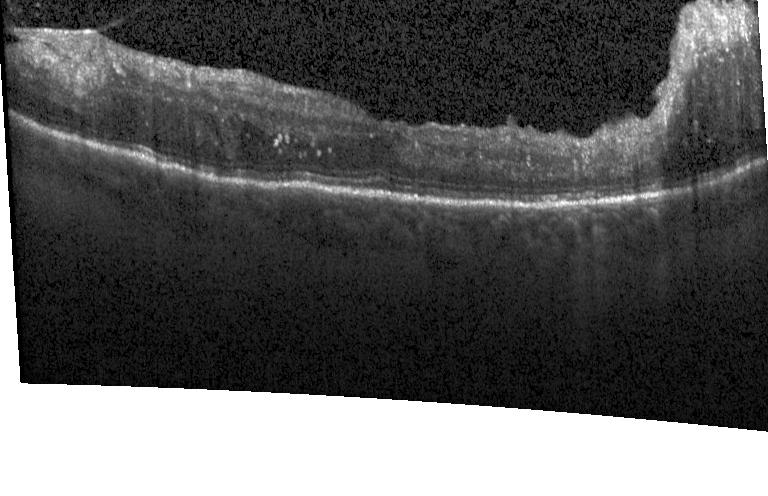
Centered on the fovea · spectral-domain OCT · instrument: Heidelberg Spectralis · OCT line scan
This B-scan demonstrates diabetic macular edema (DME).